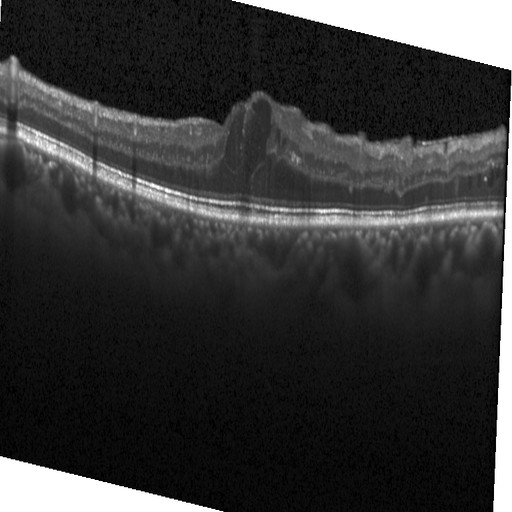
Optical coherence tomography B-scan. Instrument: Heidelberg Spectralis. Centered on the fovea. Spectral-domain optical coherence tomography.
Macular OCT: DME.